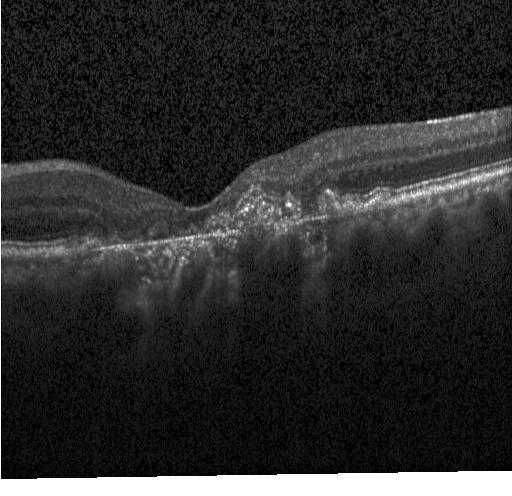
Acquired on a Heidelberg Spectralis. Spectral-domain OCT. OCT B-scan.
Diagnosis: CNV.